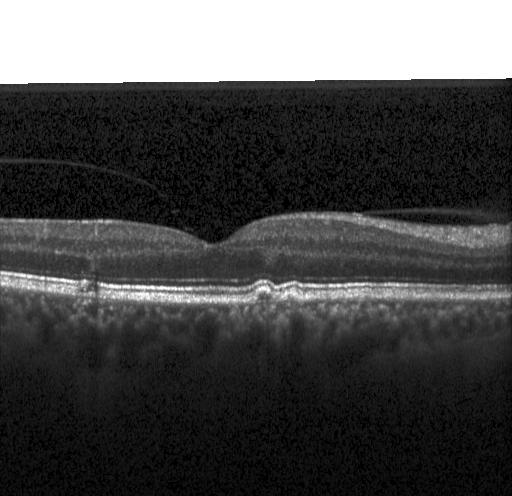

Optical coherence tomography B-scan — The scan shows multiple drusen.